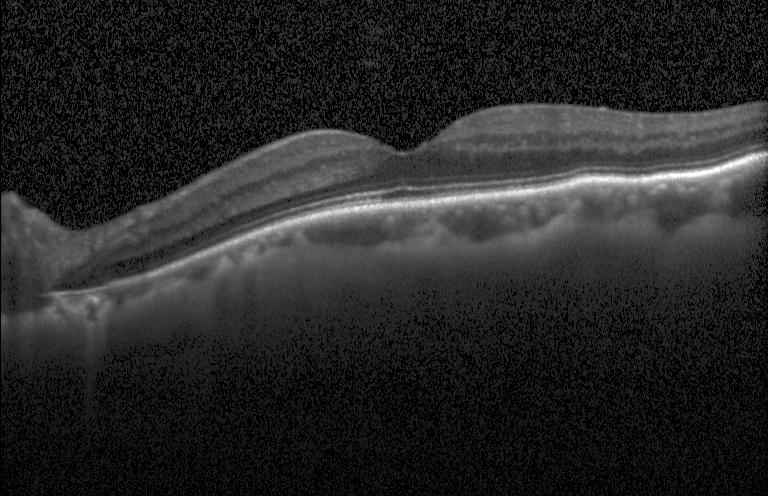 OCT B-scan showing neither CNV, DME, nor drusen.